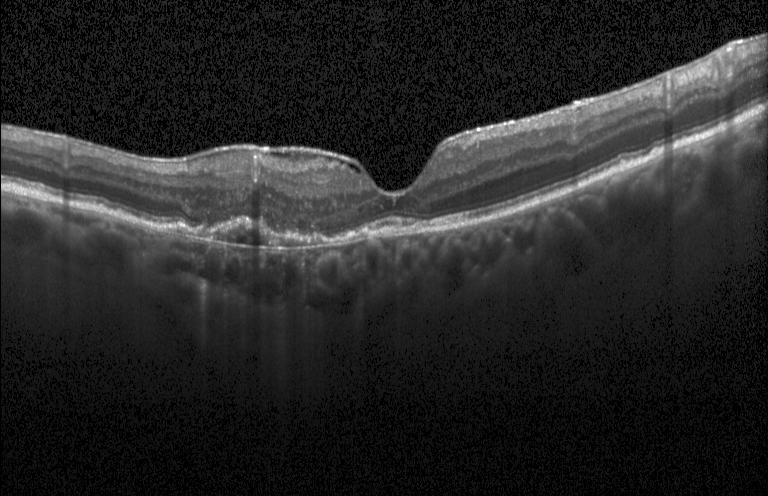 OCT B-scan showing a choroidal neovascular membrane.